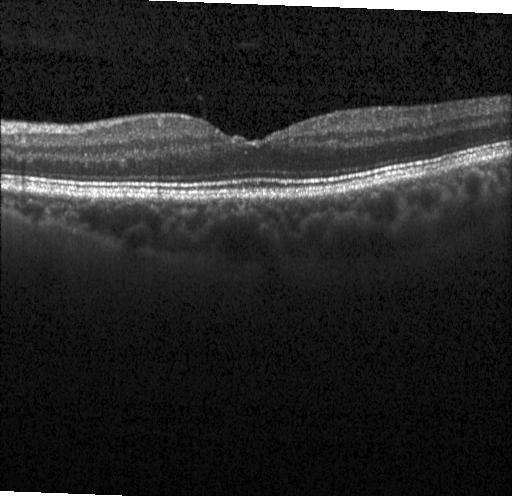
Optical coherence tomography scan
Assessment: no choroidal neovascularization, no diabetic macular edema, and no drusen.